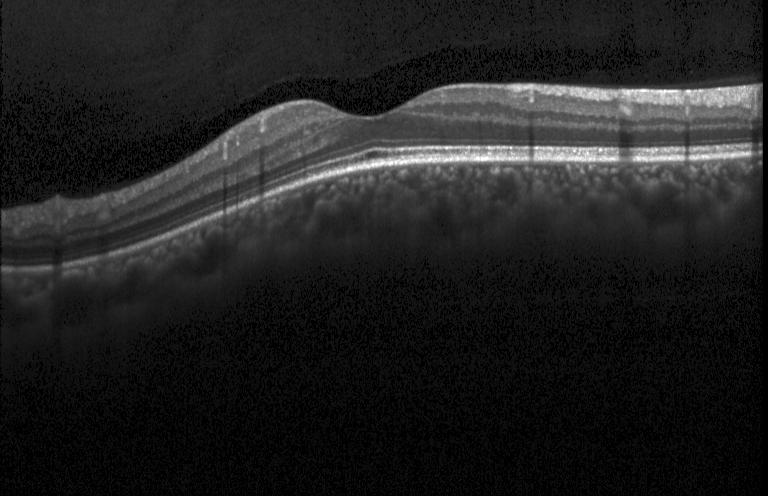

Instrument: Heidelberg Spectralis, spectral-domain OCT, OCT B-scan, macular scan. Assessment: no evidence of choroidal neovascularization, diabetic macular edema, or drusen.